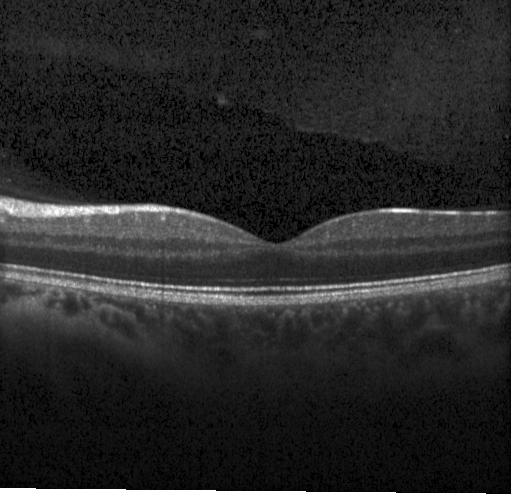 OCT scan showing no evidence of choroidal neovascularization, diabetic macular edema, or drusen.